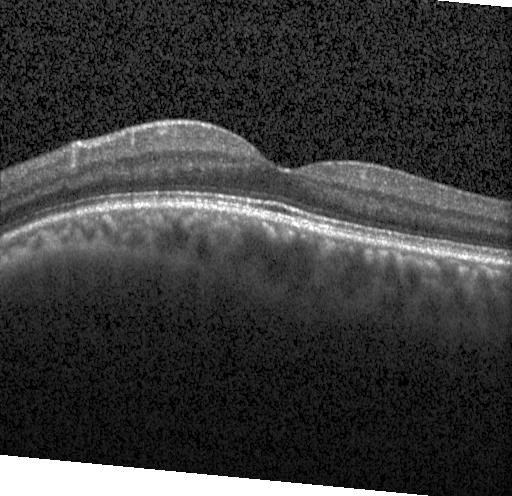
OCT finding: no choroidal neovascularization, diabetic macular edema, or drusen.